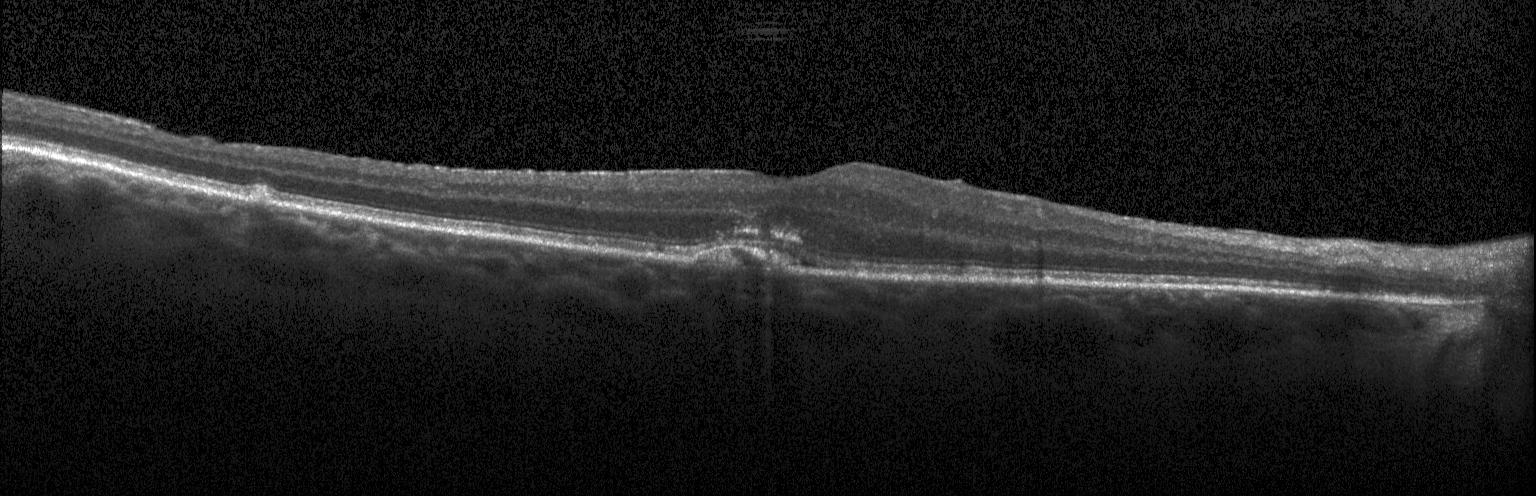

Finding: a choroidal neovascular membrane.